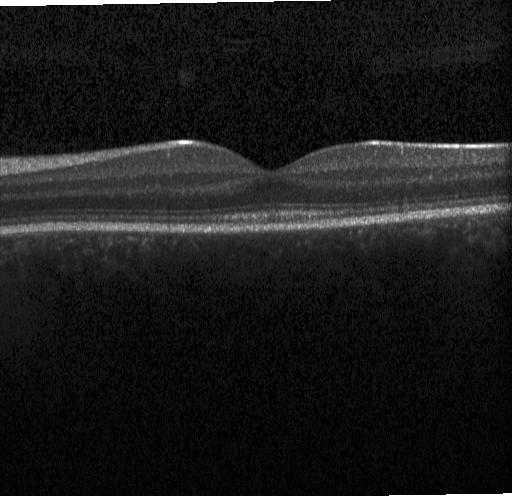 OCT B-scan; centered on the fovea. Impression: neither choroidal neovascularization, diabetic macular edema, nor drusen.